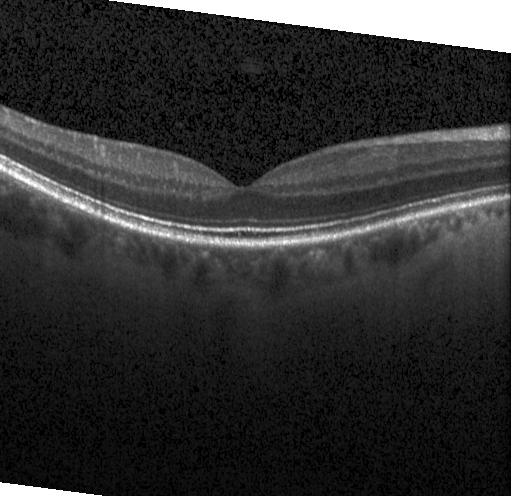
Spectral-domain optical coherence tomography, horizontal scan through the fovea, optical coherence tomography B-scan, Heidelberg Spectralis OCT system
Finding: neither choroidal neovascularization, diabetic macular edema, nor drusen.